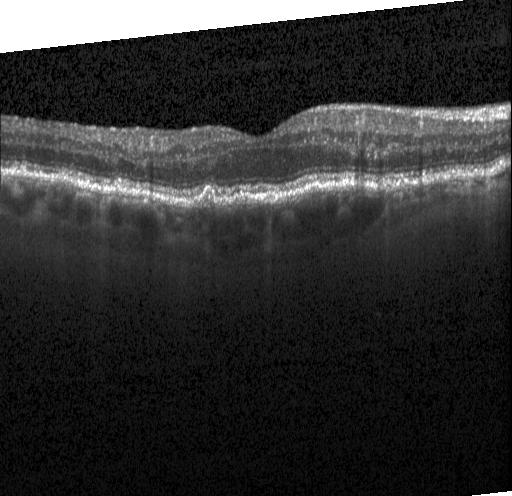 Spectral-domain OCT. Fovea-centered. Optical coherence tomography scan. Heidelberg Spectralis OCT system — Dx: drusen.